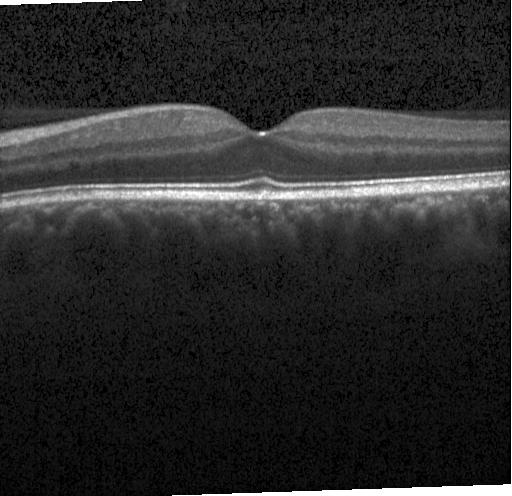 Finding: neither CNV, DME, nor drusen.